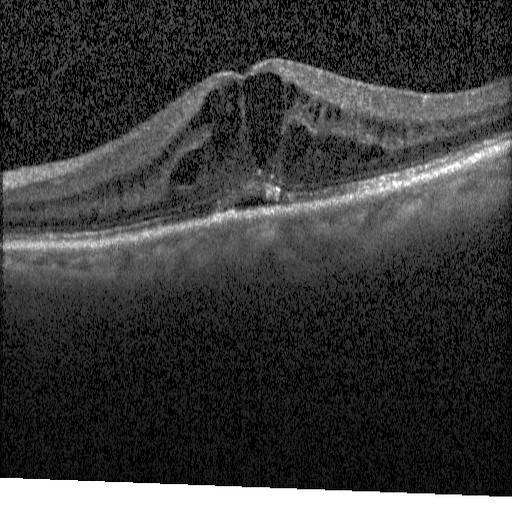 Spectral-domain optical coherence tomography · OCT B-scan — Diagnosis: diabetic macular edema (DME).